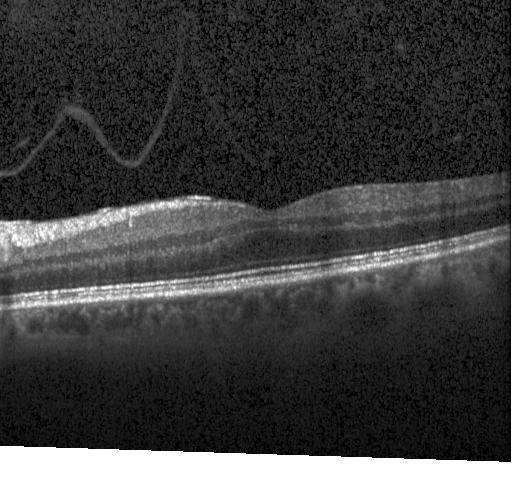

SD-OCT; OCT line scan
This B-scan demonstrates neither CNV, DME, nor drusen.